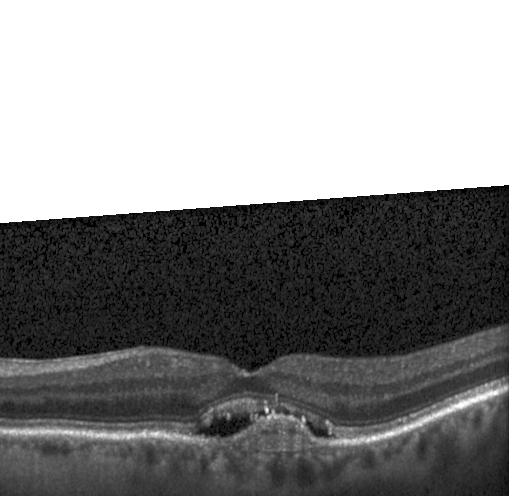

OCT line scan — Assessment: CNV.